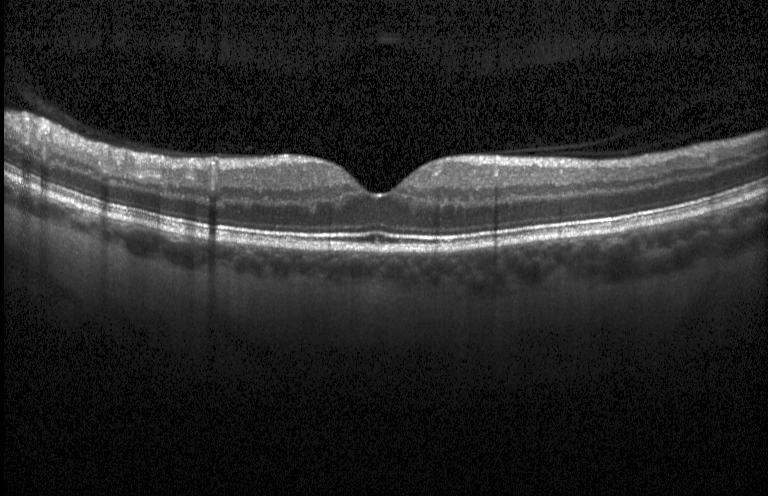

OCT B-scan, fovea-centered, spectral-domain OCT. No CNV, DME, or drusen.